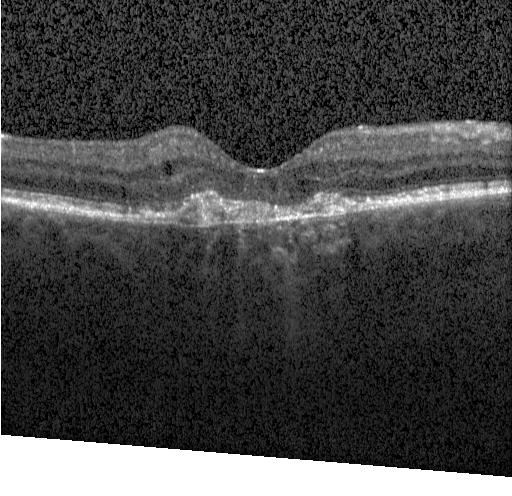 Finding: choroidal neovascularization.